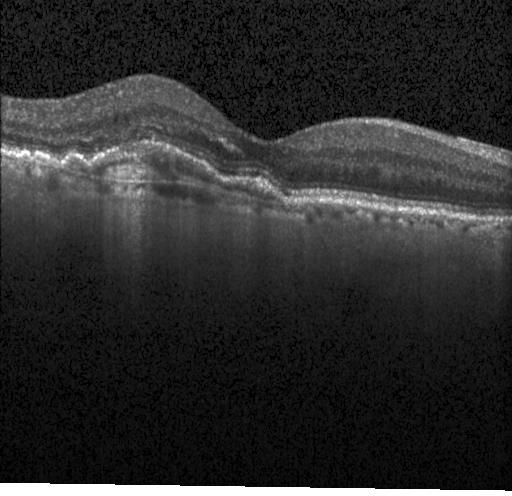

Spectral-domain optical coherence tomography · optical coherence tomography B-scan · fovea-centered. Finding: choroidal neovascularization.